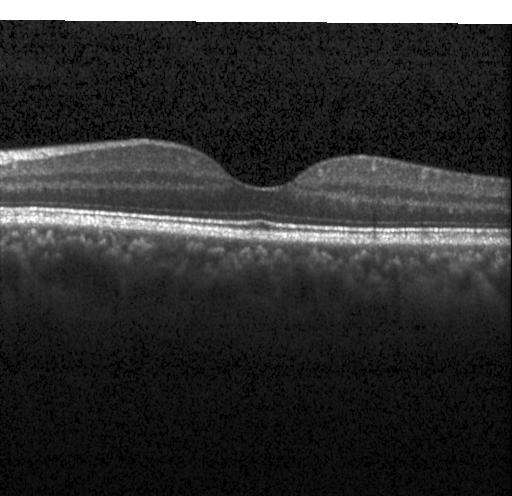 Instrument: Heidelberg Spectralis · optical coherence tomography scan. Finding: no CNV, no DME, and no drusen.